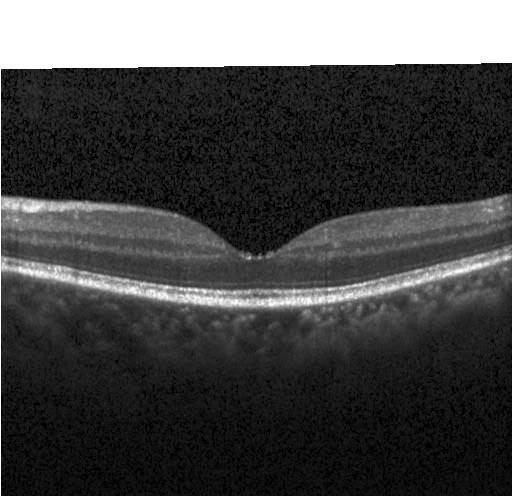 Finding: no choroidal neovascularization, diabetic macular edema, or drusen.